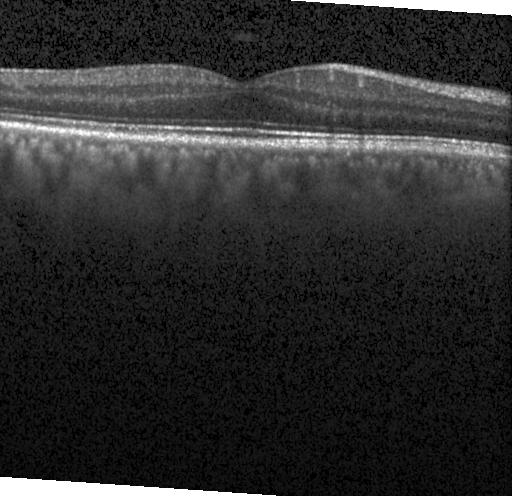
Retinal OCT cross-section. Through the macula. Heidelberg Spectralis. Assessment: no CNV, no DME, and no drusen.